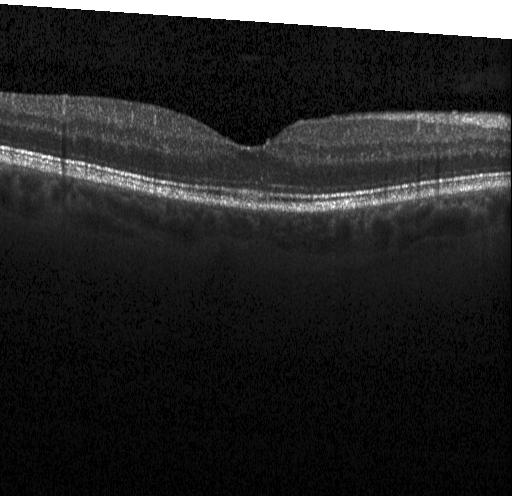
Through the macula · OCT B-scan · spectral-domain optical coherence tomography — Assessment: no evidence of choroidal neovascularization, diabetic macular edema, or drusen.